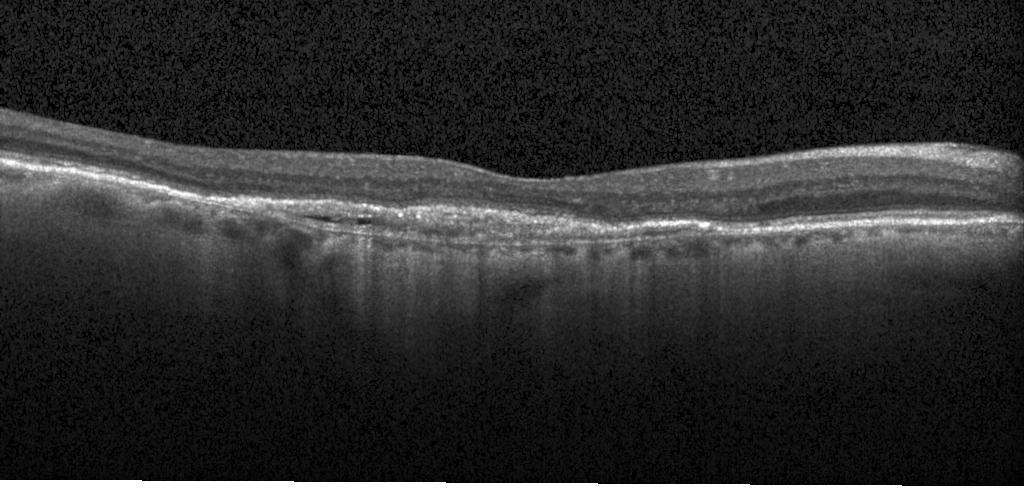 SD-OCT. Optical coherence tomography scan. Horizontal scan through the fovea. Instrument: Heidelberg Spectralis.
This B-scan demonstrates choroidal neovascularization.